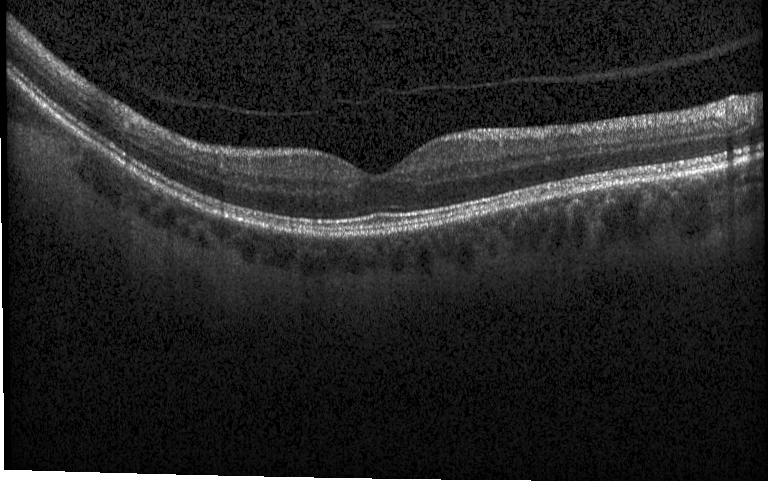 Optical coherence tomography scan — Finding: neither choroidal neovascularization, diabetic macular edema, nor drusen.